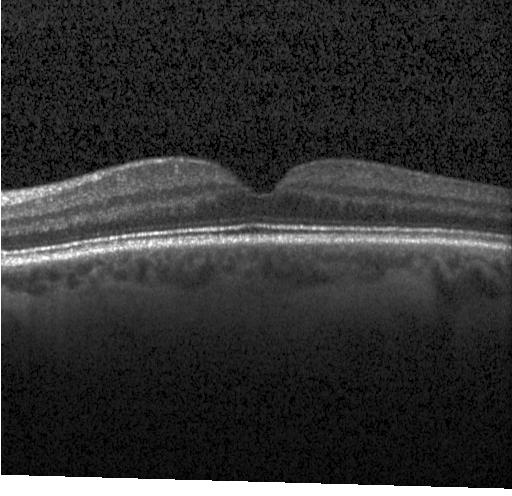 Impression: no choroidal neovascularization, diabetic macular edema, or drusen.